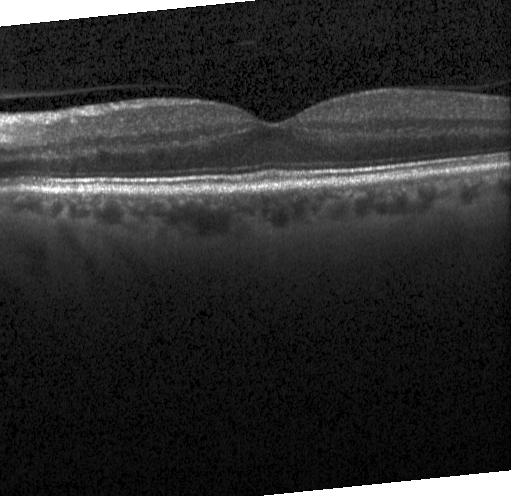
Spectral-domain OCT B-scan: no choroidal neovascularization, no diabetic macular edema, and no drusen.